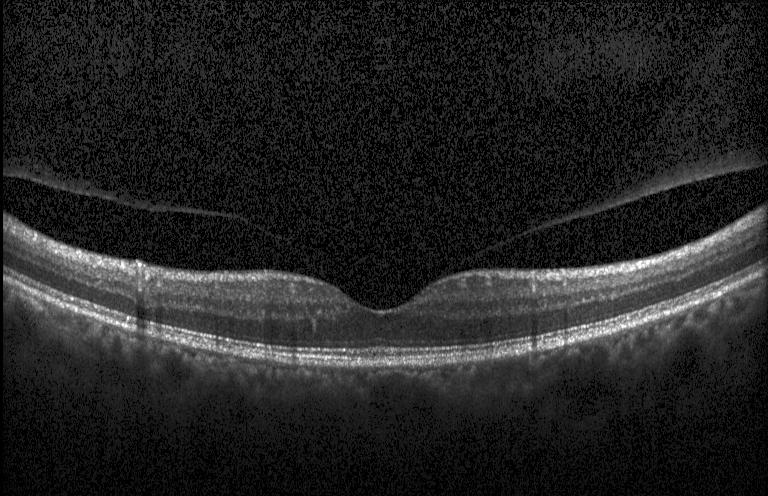 Heidelberg Spectralis OCT system, OCT B-scan.
Finding: no CNV, no DME, and no drusen.